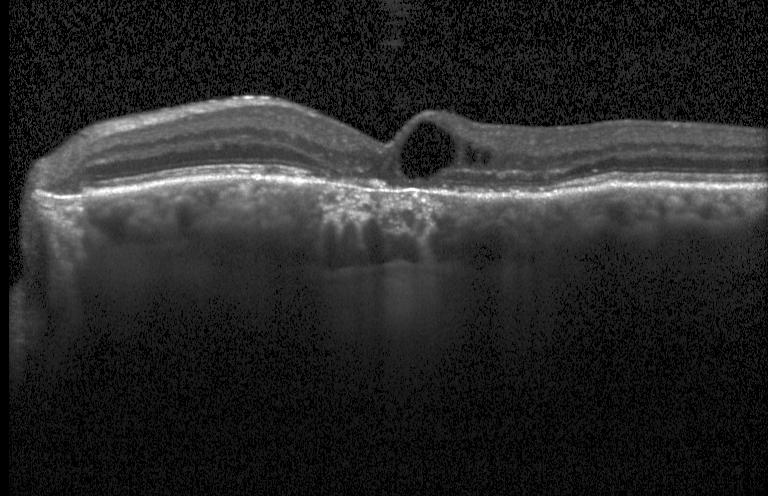

Impression: CNV.